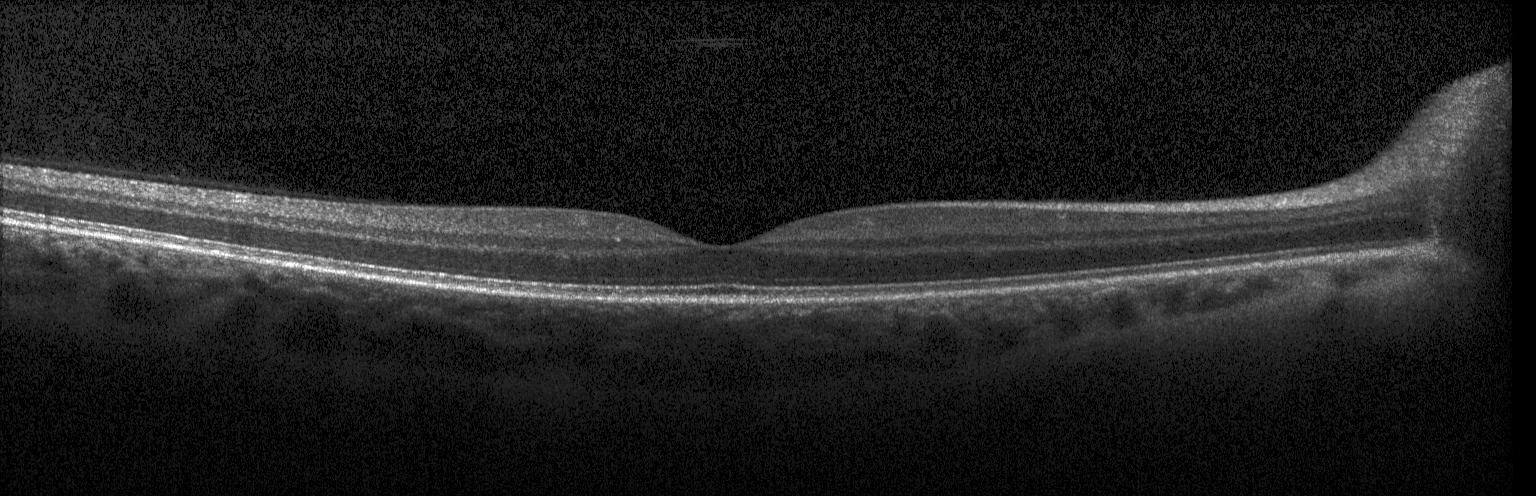

Spectral-domain optical coherence tomography, horizontal scan through the fovea, Heidelberg Spectralis, OCT B-scan.
Neither choroidal neovascularization, diabetic macular edema, nor drusen.